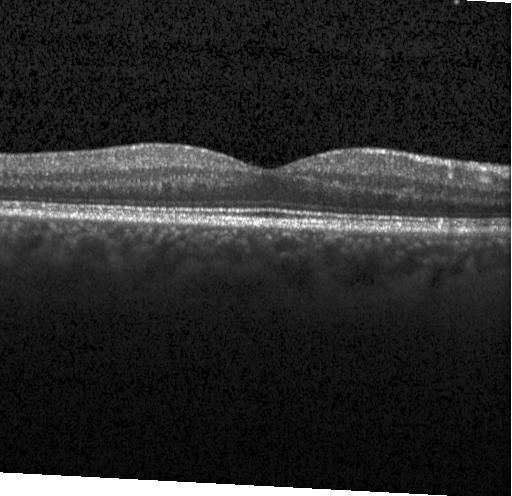 Impression: no evidence of choroidal neovascularization, diabetic macular edema, or drusen.